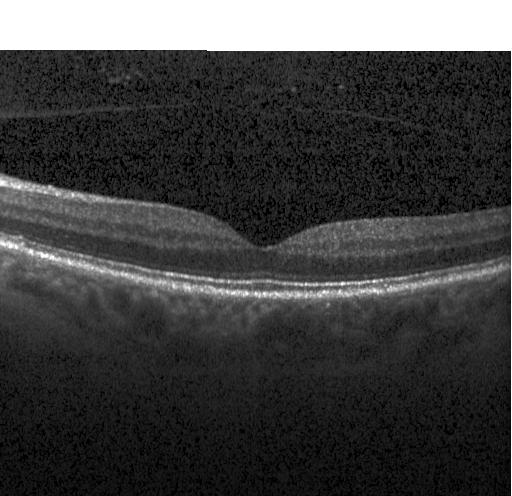

Diagnosis: no evidence of CNV, DME, or drusen.